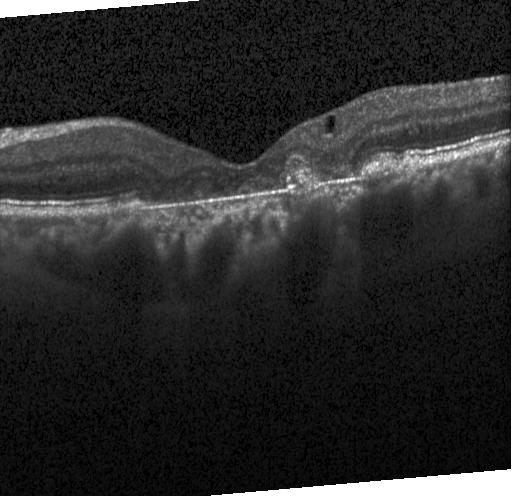
Optical coherence tomography B-scan
Dx: a choroidal neovascular membrane.